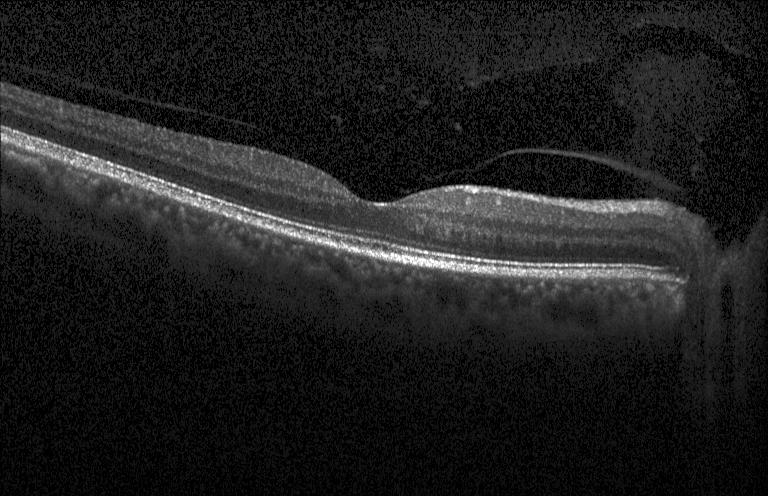

Optical coherence tomography B-scan. Acquired on a Heidelberg Spectralis. Spectral-domain OCT. Fovea-centered — Diagnosis: no evidence of CNV, DME, or drusen.